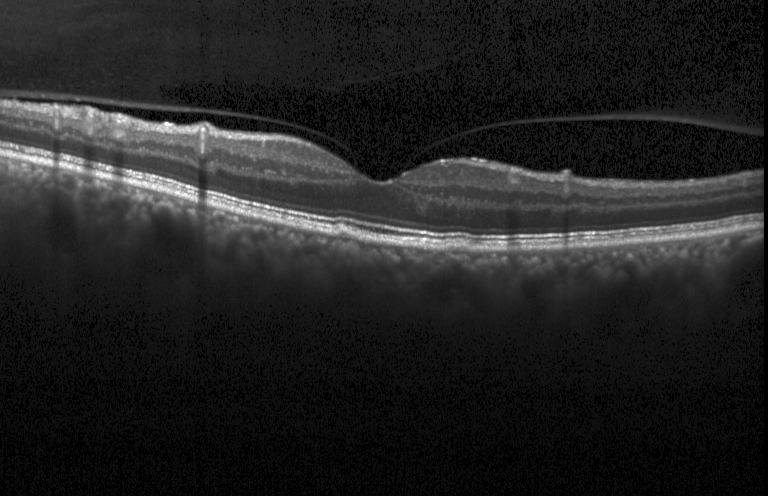
Macular OCT demonstrating drusen.